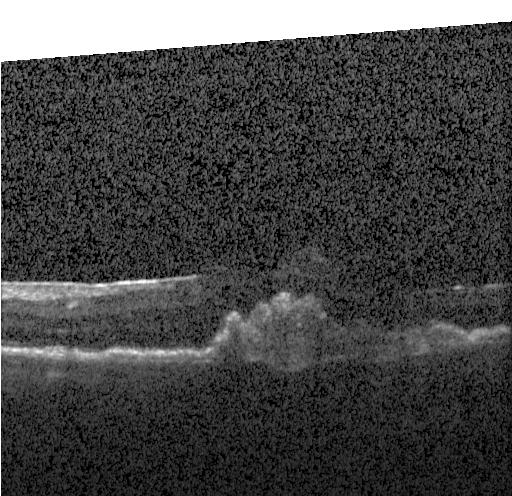

Diagnosis: a choroidal neovascular membrane.